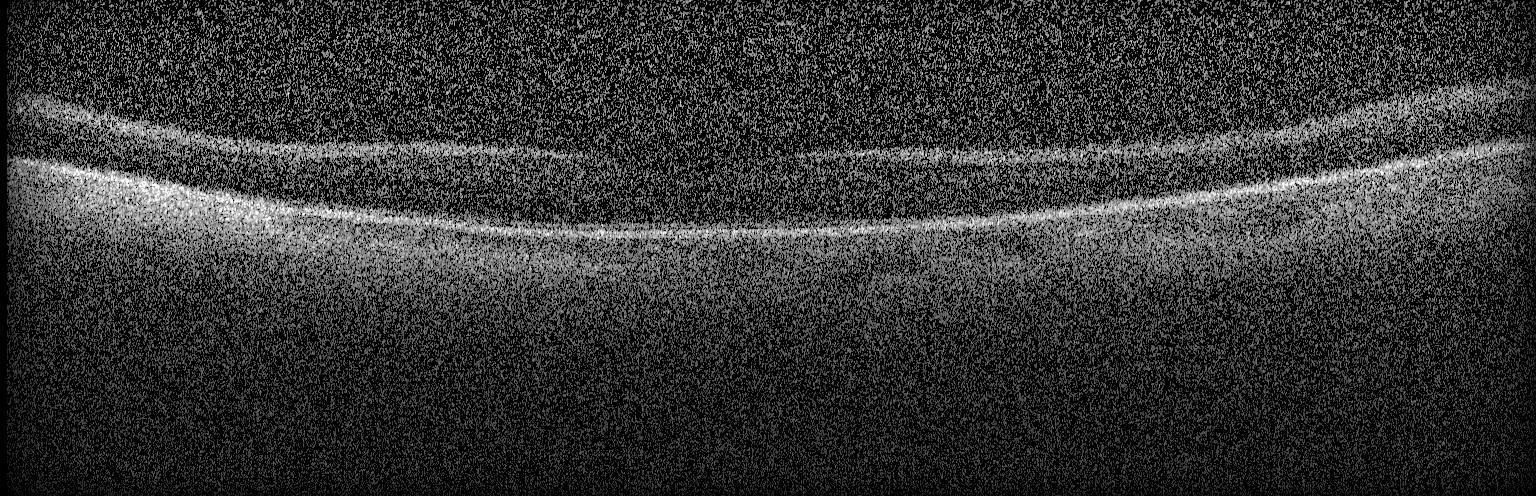

Optical coherence tomography scan — Neither choroidal neovascularization, diabetic macular edema, nor drusen.